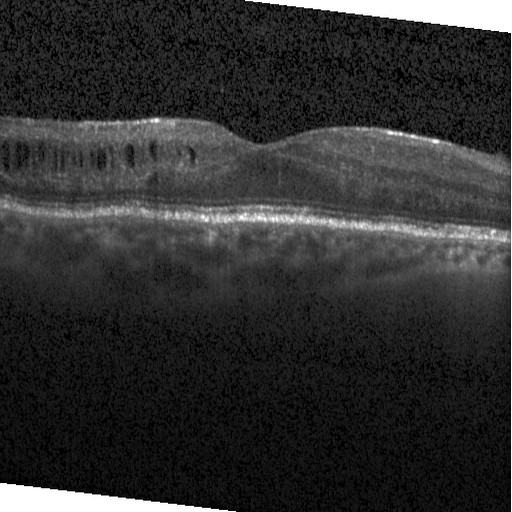 Diagnosis: diabetic macular edema (DME).